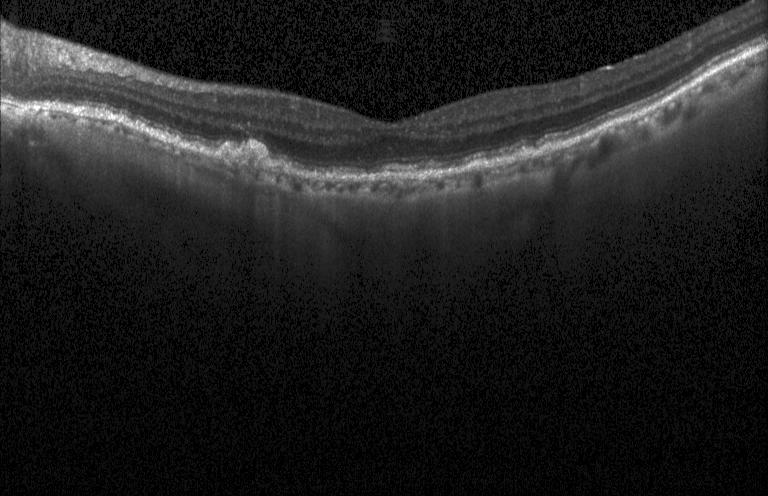 Spectral-domain optical coherence tomography. Retinal OCT cross-section. Fovea-centered — Diagnosis: choroidal neovascularization.